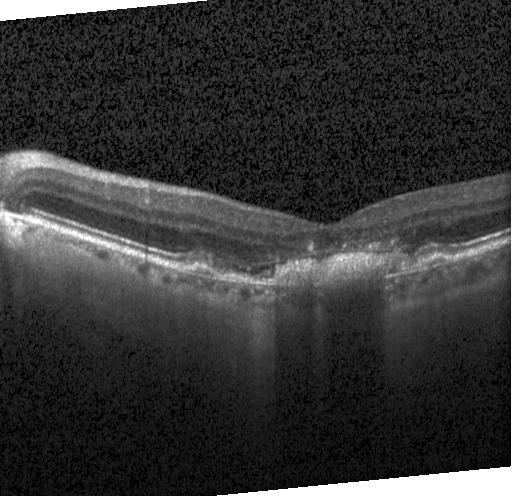 Retinal OCT B-scan. Diagnosis: choroidal neovascularization (CNV).